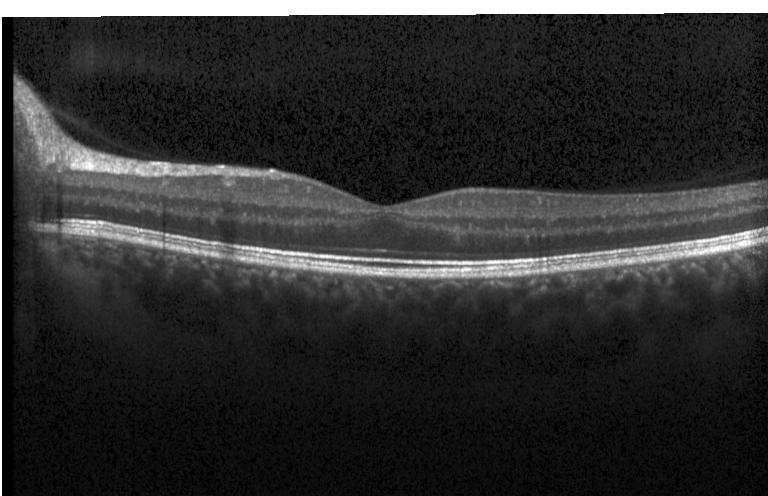 Retinal OCT cross-section, spectral-domain optical coherence tomography, through the macula, acquired on a Heidelberg Spectralis. Finding: no choroidal neovascularization, diabetic macular edema, or drusen.